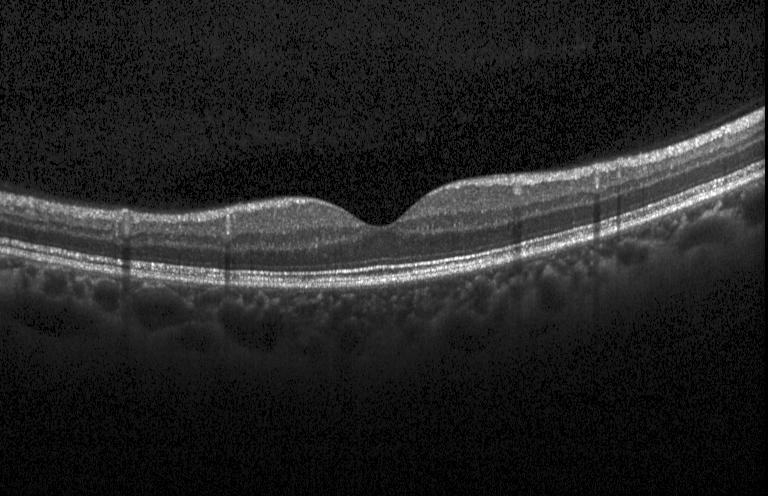 Impression: no evidence of CNV, DME, or drusen.